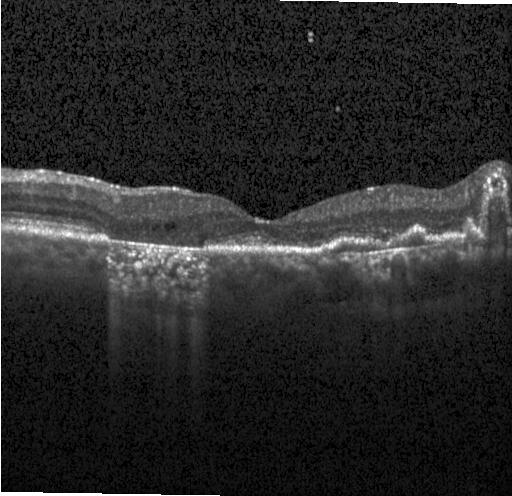
OCT line scan, horizontal scan through the fovea. Finding: a choroidal neovascular membrane.